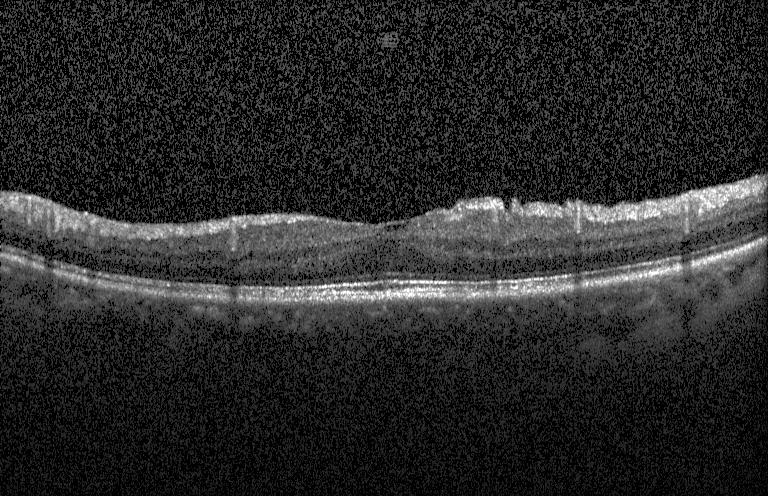 Optical coherence tomography B-scan
Impression: neither choroidal neovascularization, diabetic macular edema, nor drusen.